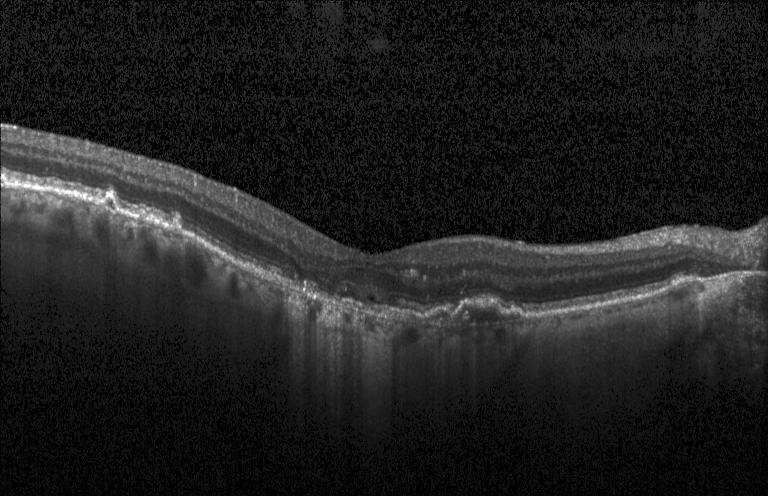

Optical coherence tomography scan · centered on the fovea — CNV.